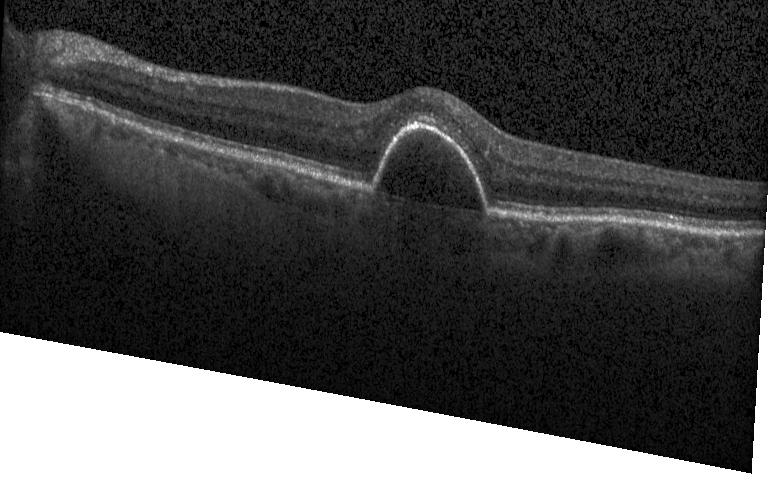

Retinal OCT cross-section, acquired on a Heidelberg Spectralis, spectral-domain OCT. Diagnosis: CNV.